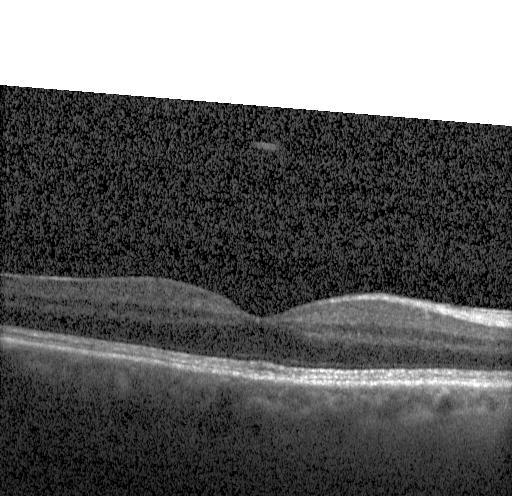

Fovea-centered. Spectral-domain OCT. Retinal OCT B-scan — Diagnosis: no choroidal neovascularization, no diabetic macular edema, and no drusen.